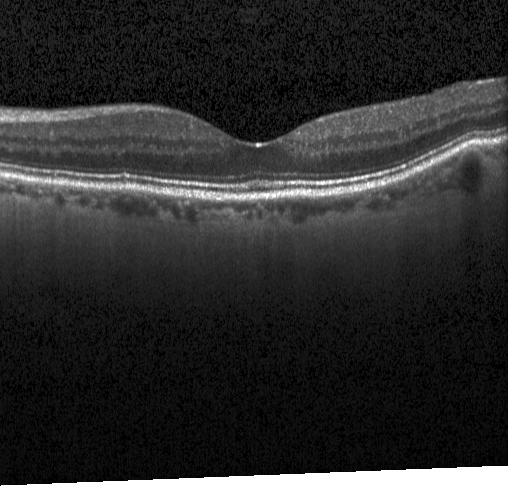

Diagnosis: no choroidal neovascularization, diabetic macular edema, or drusen.